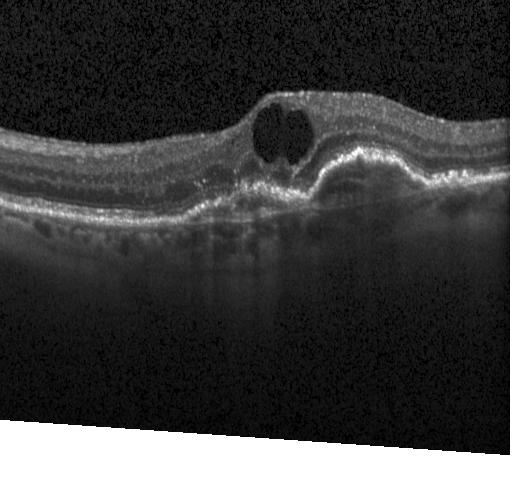
Retinal OCT B-scan
Impression: a choroidal neovascular membrane.